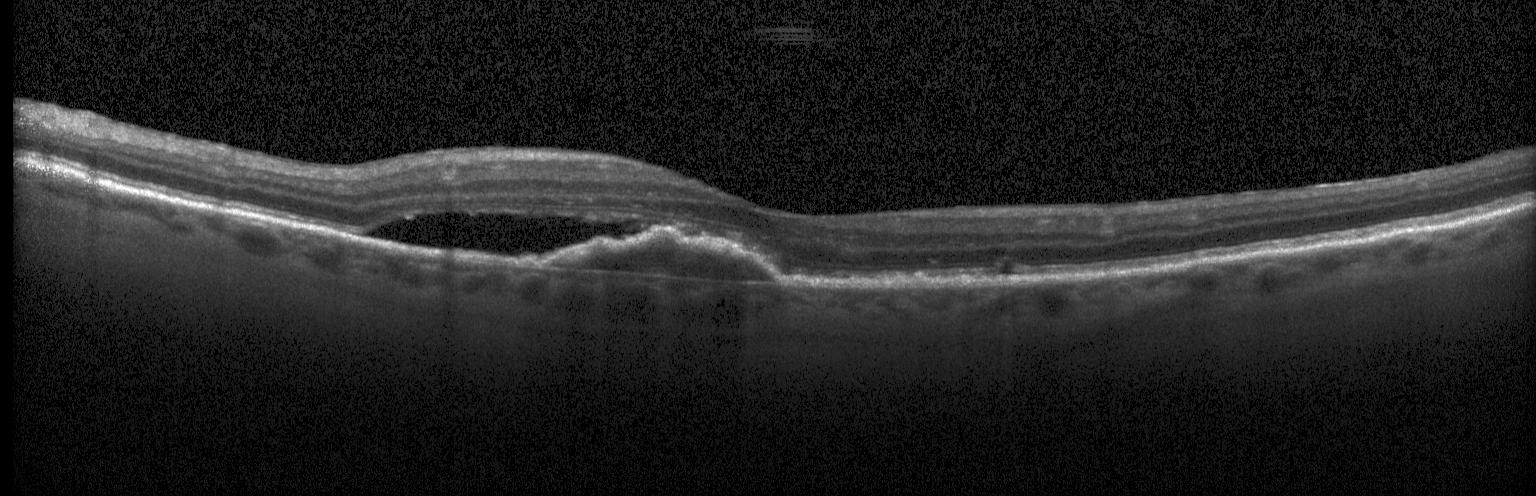 Optical coherence tomography B-scan — Assessment: a choroidal neovascular membrane.